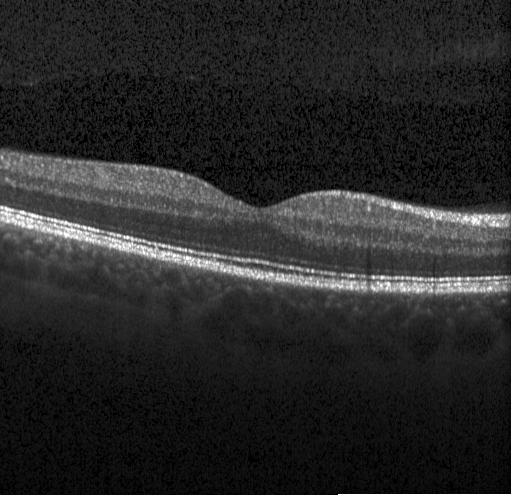
OCT B-scan showing neither choroidal neovascularization, diabetic macular edema, nor drusen.